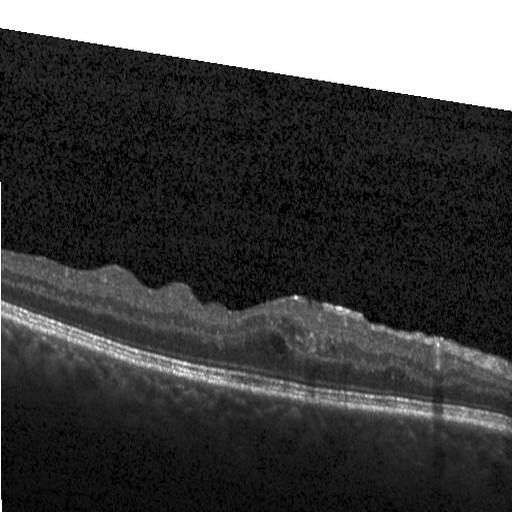 Finding: diabetic macular edema (DME).